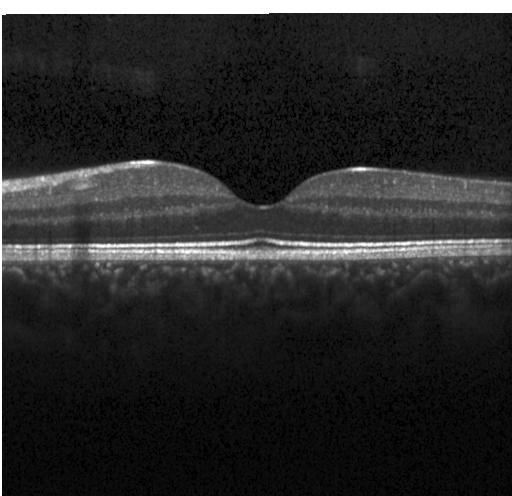

Diagnosis: no CNV, DME, or drusen.